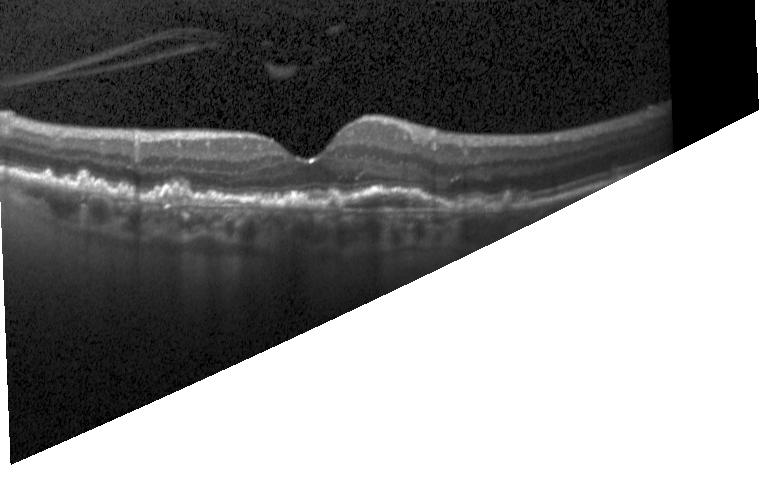

Retinal OCT B-scan — OCT finding: CNV.